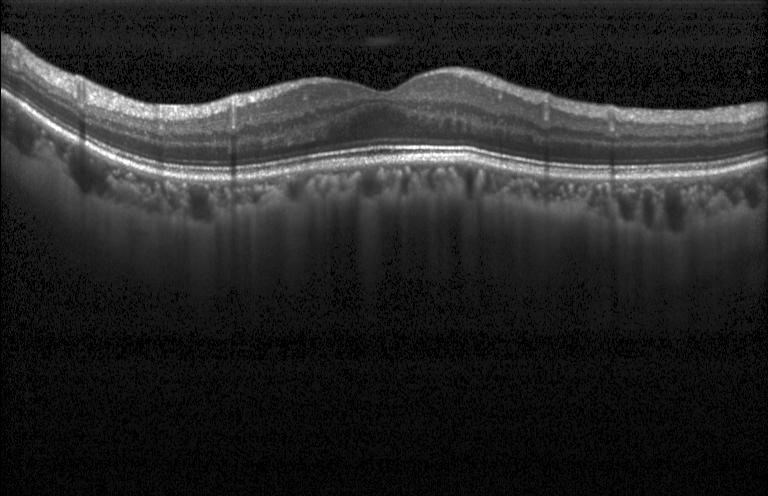

No evidence of choroidal neovascularization, diabetic macular edema, or drusen.